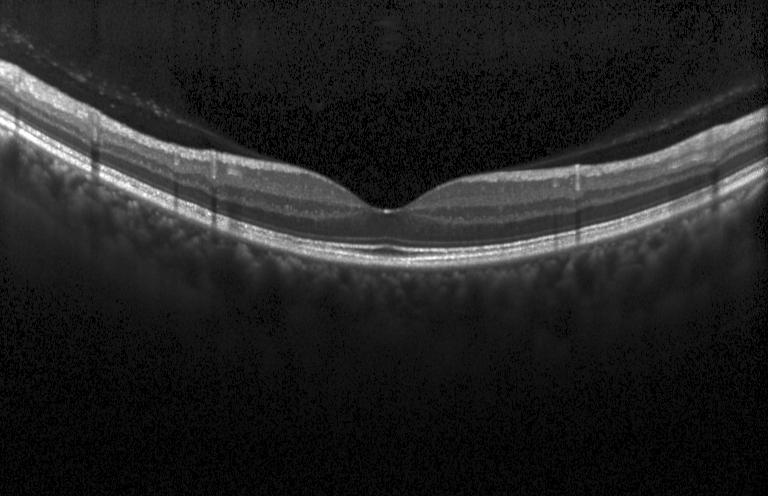

No choroidal neovascularization, diabetic macular edema, or drusen.